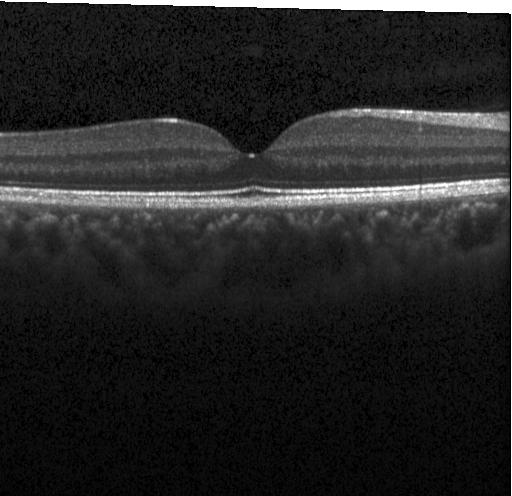
Heidelberg Spectralis, OCT line scan, fovea-centered
Macular OCT: no CNV, no DME, and no drusen.